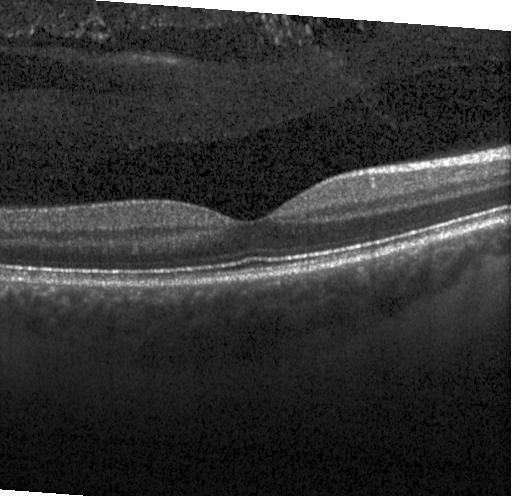

OCT line scan; spectral-domain optical coherence tomography; instrument: Heidelberg Spectralis — Diagnosis: no CNV, no DME, and no drusen.